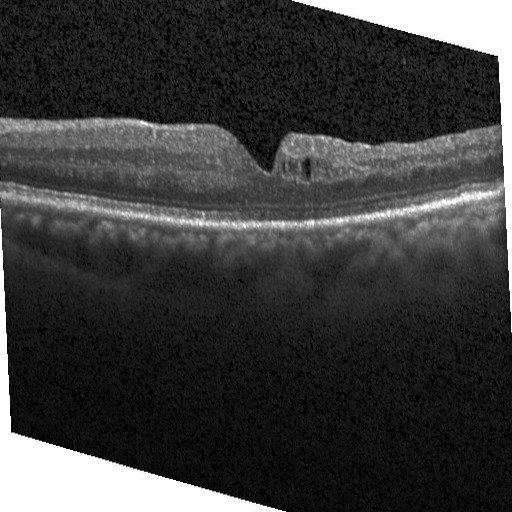
OCT line scan — Finding: diabetic macular edema (DME).